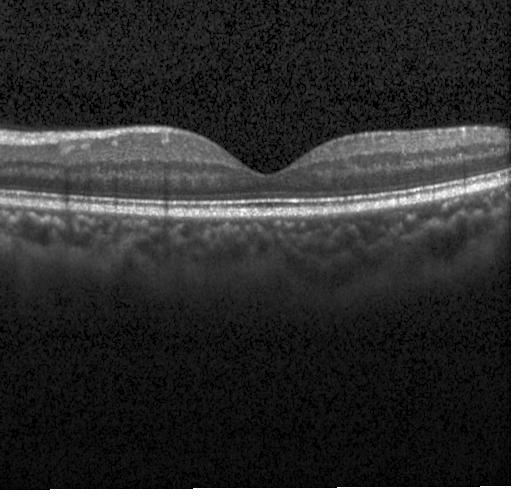

Impression: no evidence of choroidal neovascularization, diabetic macular edema, or drusen.